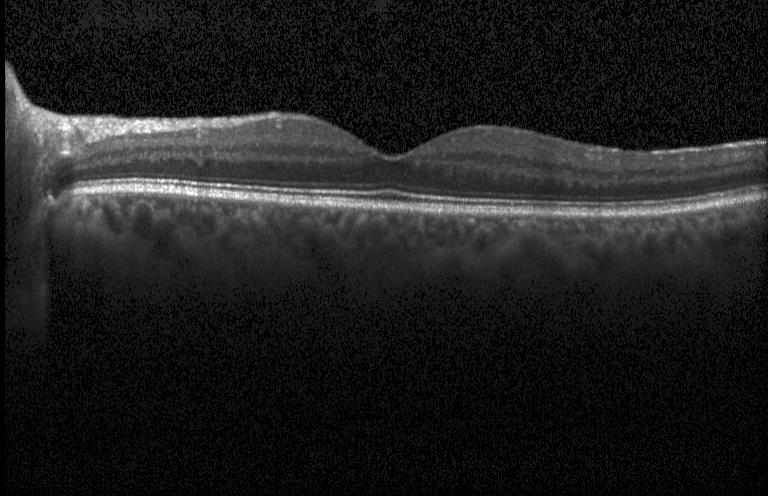

Spectral-domain OCT; Heidelberg Spectralis; retinal OCT B-scan. Impression: no CNV, DME, or drusen.